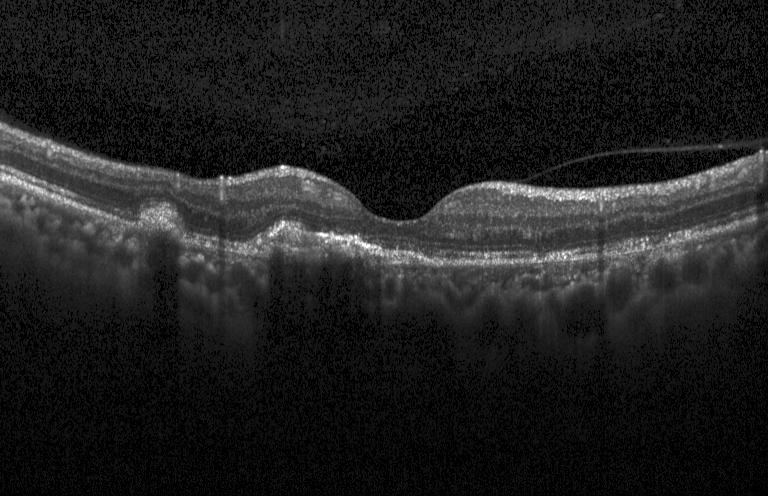
Optical coherence tomography B-scan.
Assessment: a choroidal neovascular membrane.